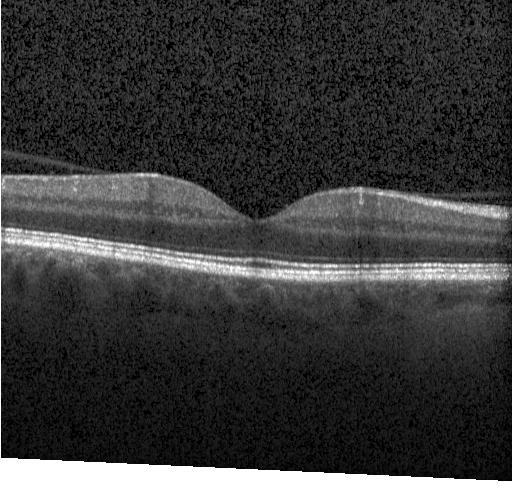 SD-OCT, optical coherence tomography scan, acquired on a Heidelberg Spectralis, fovea-centered. The scan shows no evidence of choroidal neovascularization, diabetic macular edema, or drusen.